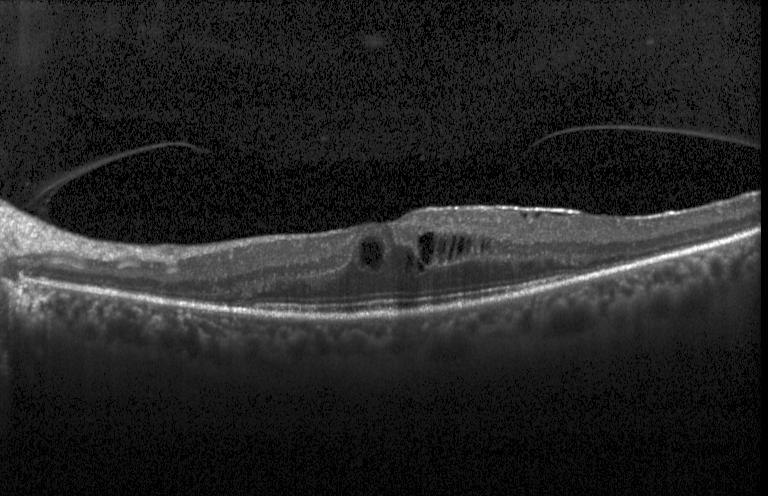
Spectral-domain OCT. Retinal OCT B-scan. Instrument: Heidelberg Spectralis. Fovea-centered.
Assessment: diabetic macular edema (DME).